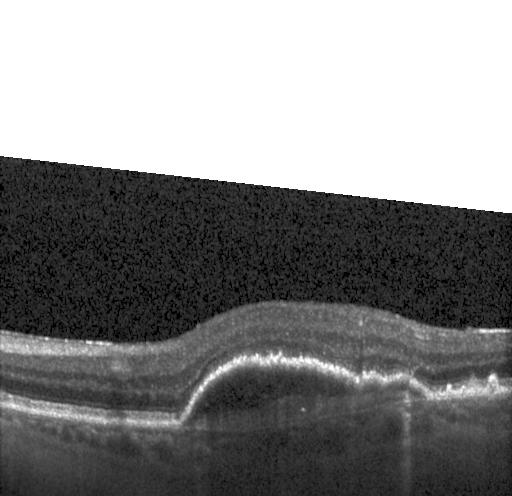

Optical coherence tomography scan · SD-OCT.
Assessment: CNV.